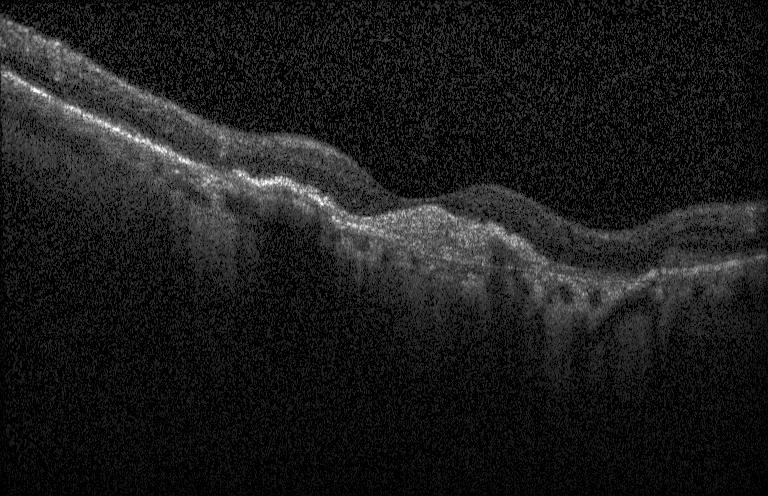
Retinal OCT cross-section. Choroidal neovascularization (CNV).